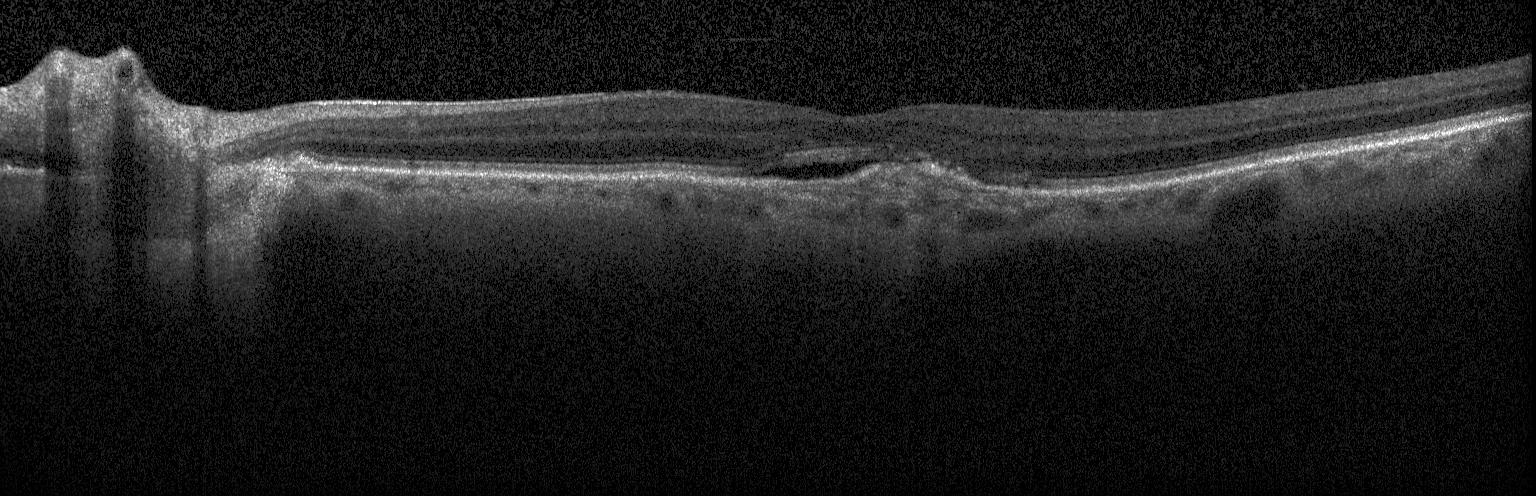
OCT B-scan, acquired on a Heidelberg Spectralis, macular scan, spectral-domain OCT.
Finding: CNV.